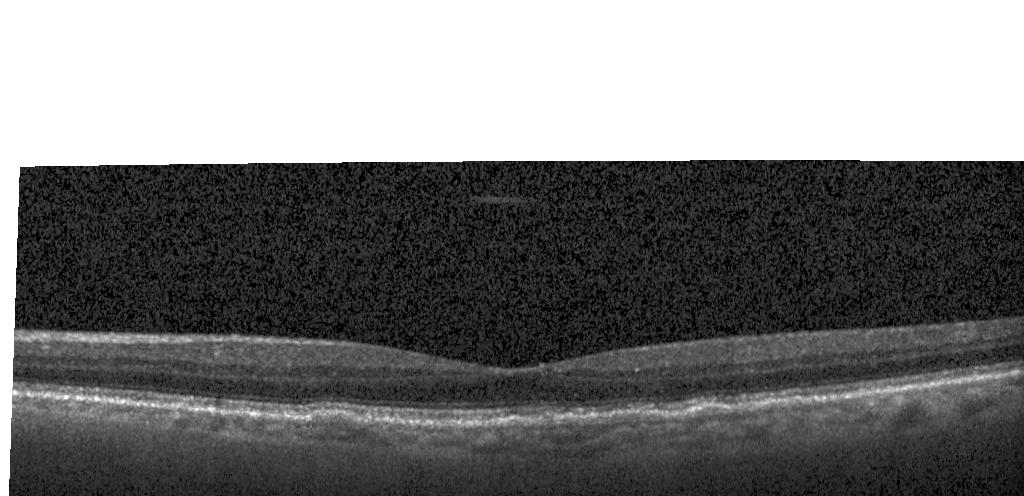 Instrument: Heidelberg Spectralis; retinal OCT cross-section; fovea-centered; SD-OCT.
Dx: sub-RPE drusenoid deposits.